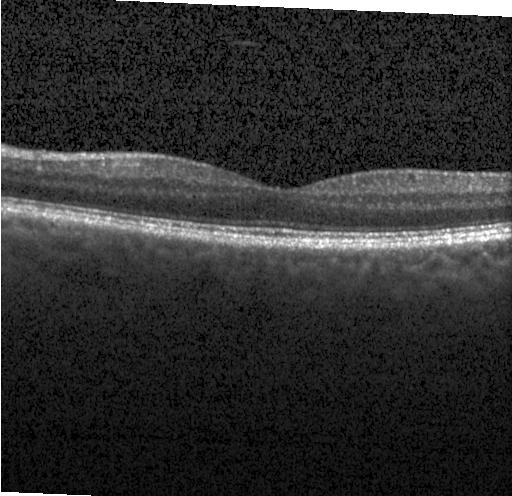
Diagnosis: no choroidal neovascularization, diabetic macular edema, or drusen.